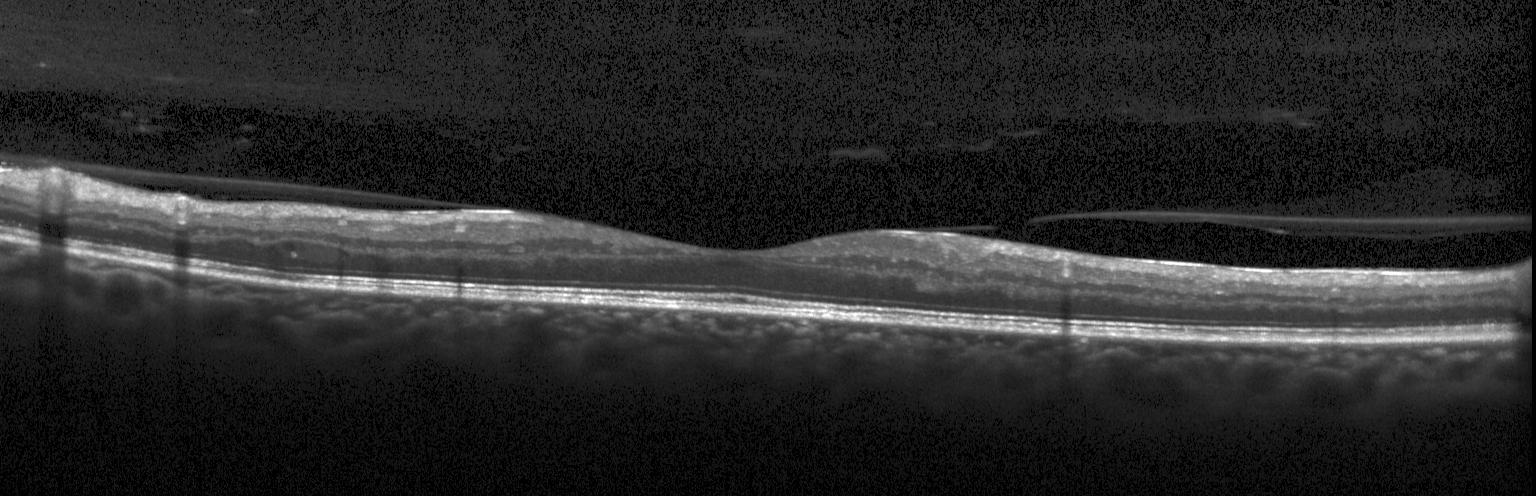

Optical coherence tomography B-scan; Heidelberg Spectralis.
Assessment: no evidence of CNV, DME, or drusen.